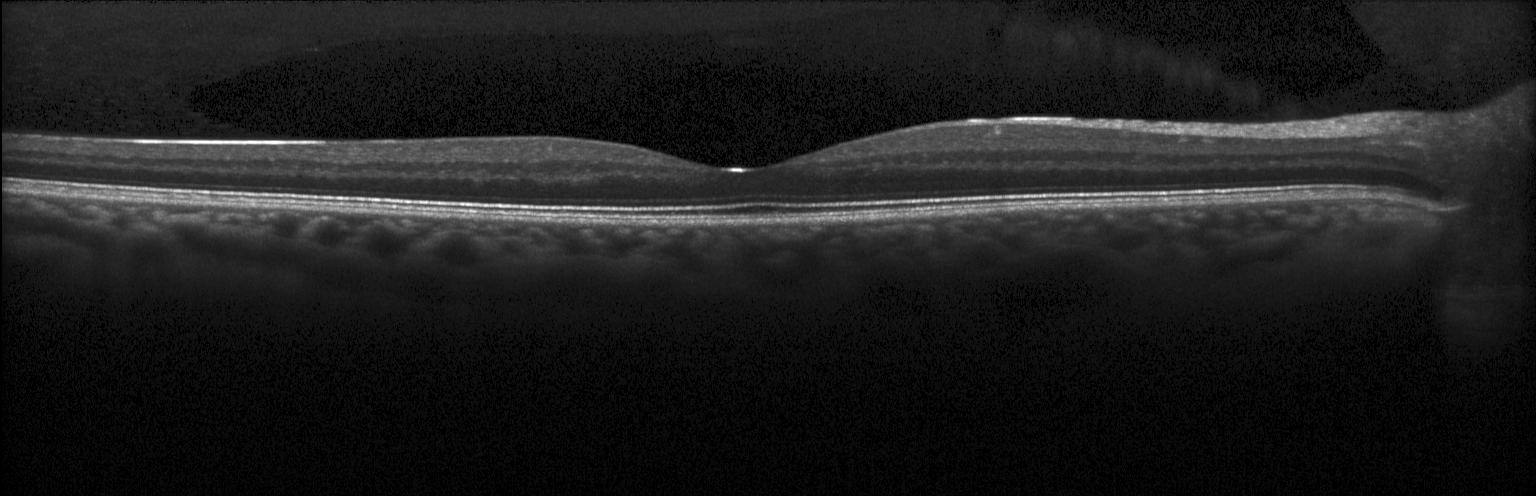

Retinal OCT B-scan. Dx: no choroidal neovascularization, no diabetic macular edema, and no drusen.